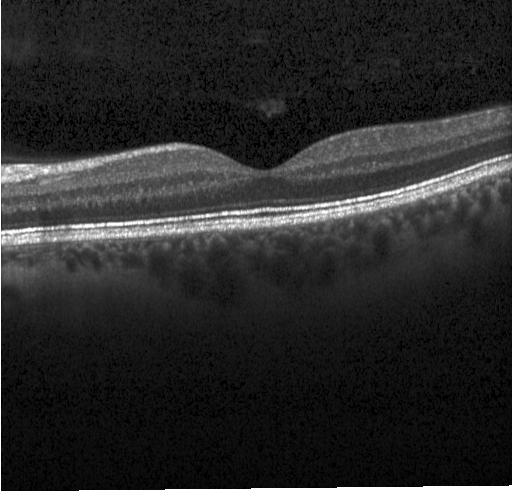

Heidelberg Spectralis OCT system. OCT line scan — No evidence of choroidal neovascularization, diabetic macular edema, or drusen.